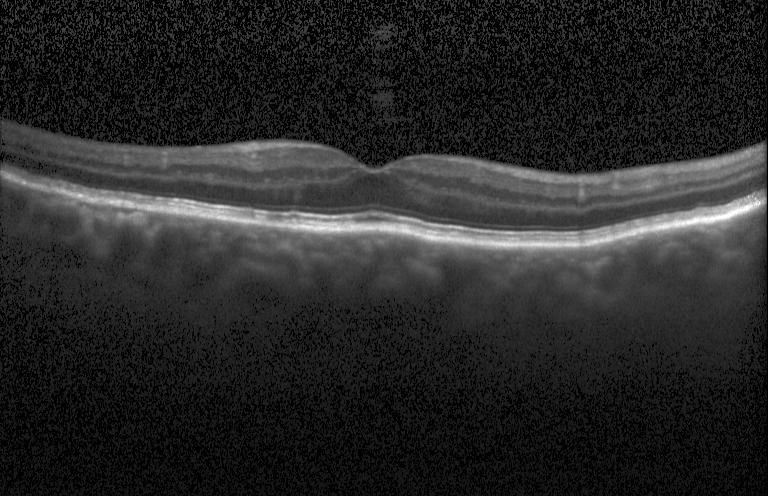 Fovea-centered, instrument: Heidelberg Spectralis, spectral-domain optical coherence tomography, retinal OCT cross-section.
This B-scan demonstrates neither choroidal neovascularization, diabetic macular edema, nor drusen.